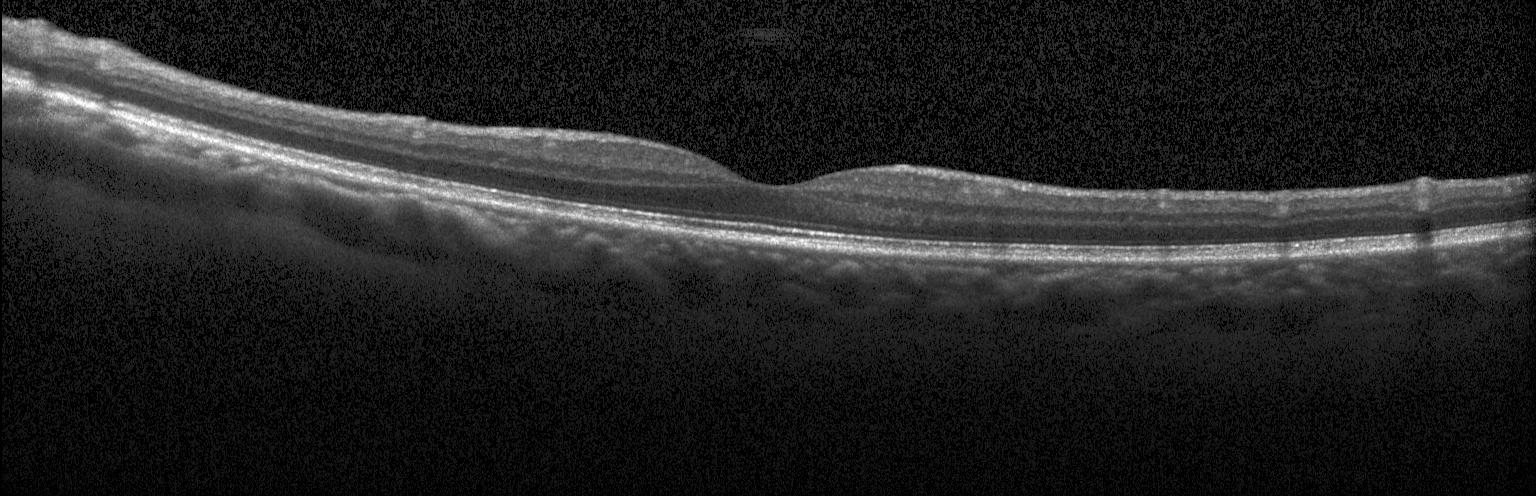
Dx: no choroidal neovascularization, diabetic macular edema, or drusen.